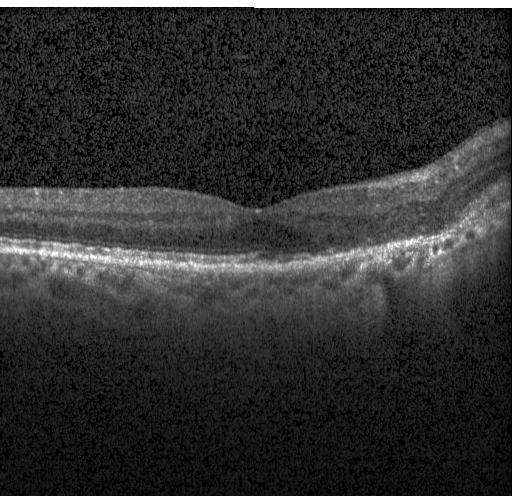 Retinal OCT B-scan; spectral-domain optical coherence tomography — Diagnosis: a choroidal neovascular membrane.